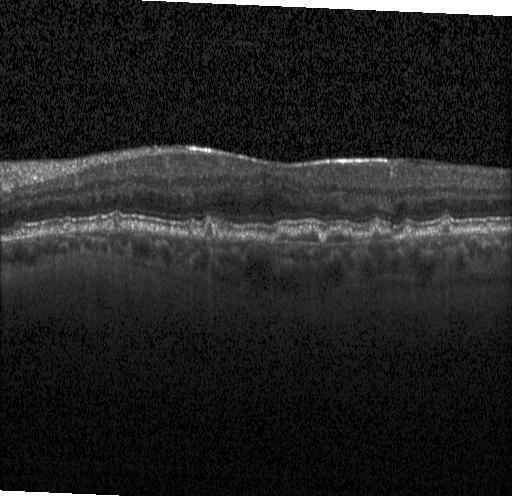

Optical coherence tomography scan
This B-scan demonstrates sub-RPE drusenoid deposits.